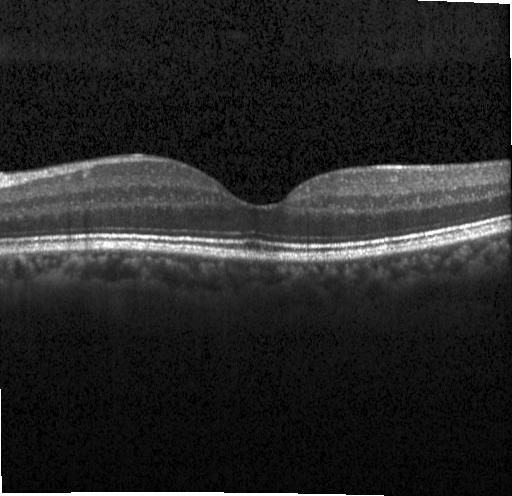
Spectral-domain optical coherence tomography · OCT B-scan · acquired on a Heidelberg Spectralis · fovea-centered — Impression: no choroidal neovascularization, diabetic macular edema, or drusen.